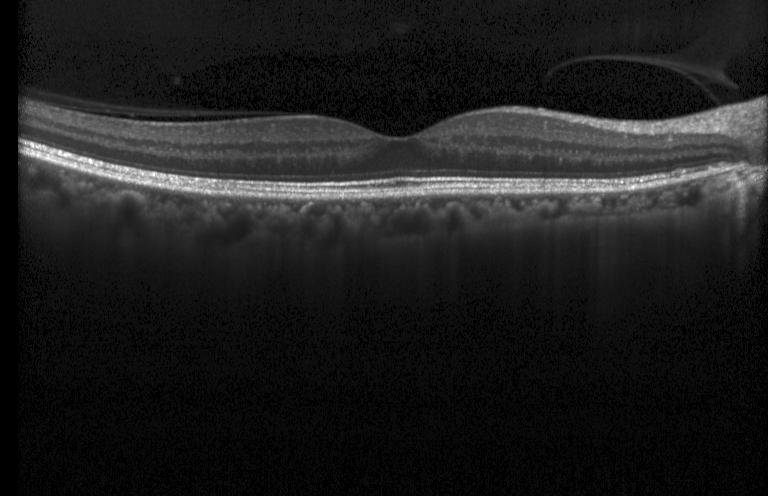

This B-scan demonstrates neither choroidal neovascularization, diabetic macular edema, nor drusen.